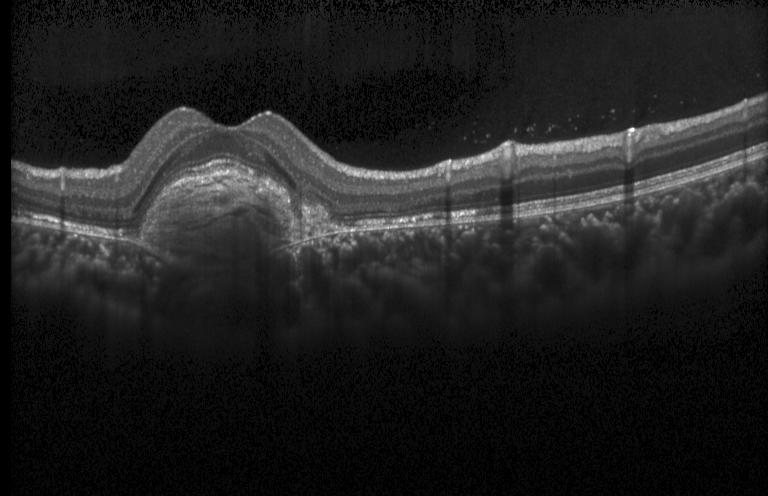
Spectral-domain OCT B-scan: choroidal neovascularization (CNV).